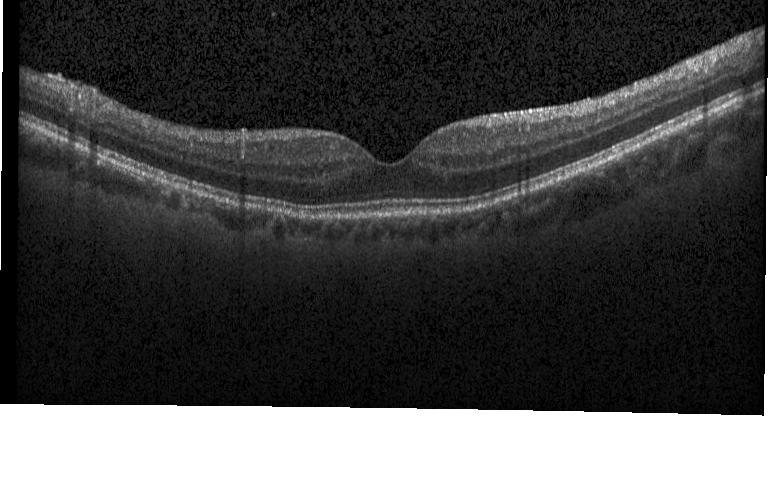

SD-OCT; acquired on a Heidelberg Spectralis; centered on the fovea; retinal OCT cross-section.
Impression: neither choroidal neovascularization, diabetic macular edema, nor drusen.